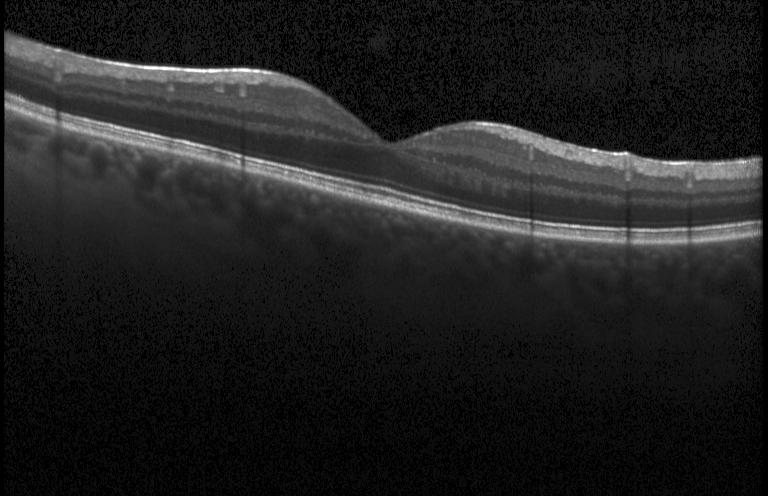
Macular scan; OCT B-scan; Heidelberg Spectralis; spectral-domain optical coherence tomography
Finding: no evidence of choroidal neovascularization, diabetic macular edema, or drusen.